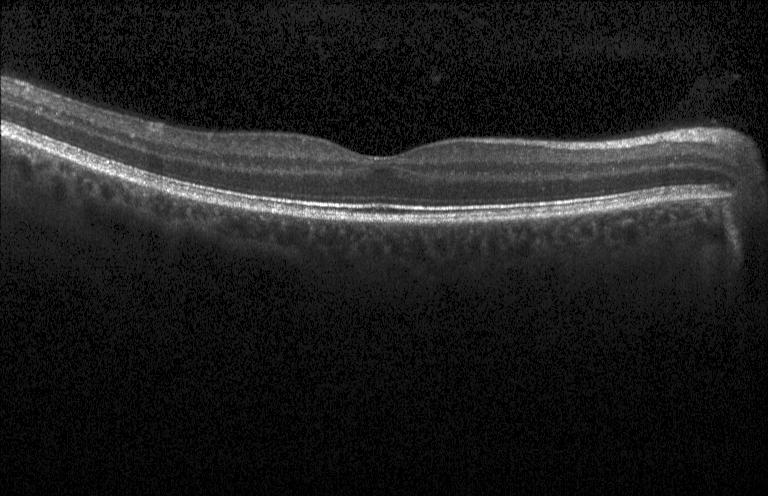
Spectral-domain optical coherence tomography. OCT B-scan. Macular scan
This B-scan demonstrates no choroidal neovascularization, no diabetic macular edema, and no drusen.